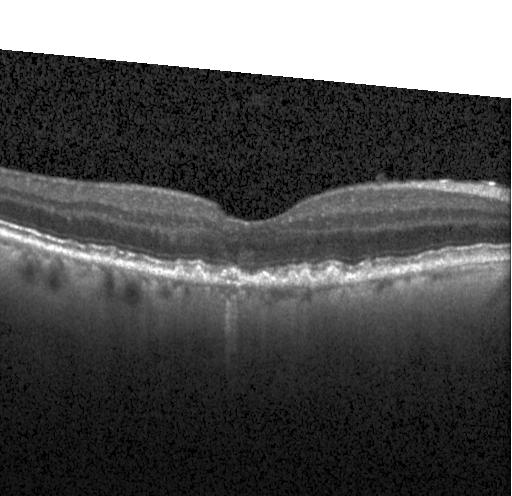 This B-scan demonstrates sub-RPE drusenoid deposits.